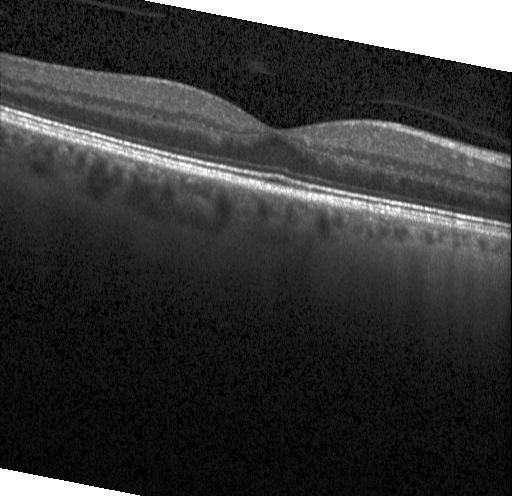 Optical coherence tomography B-scan · Heidelberg Spectralis — The scan shows no CNV, no DME, and no drusen.